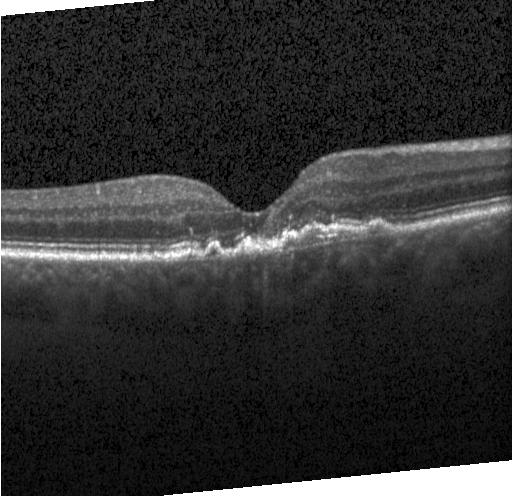 Spectral-domain OCT B-scan: choroidal neovascularization (CNV).